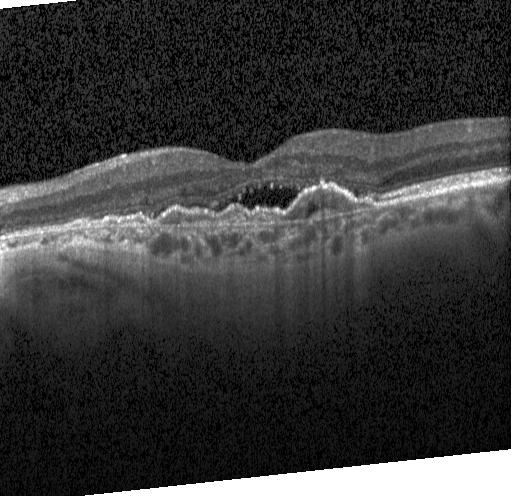

Retinal OCT cross-section showing a choroidal neovascular membrane.